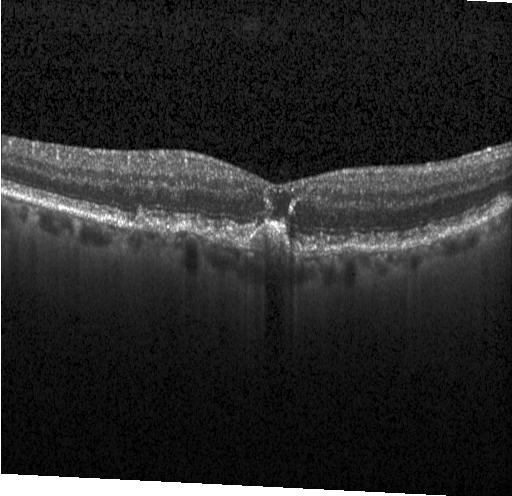

Retinal OCT B-scan · spectral-domain optical coherence tomography.
Finding: sub-RPE drusenoid deposits.